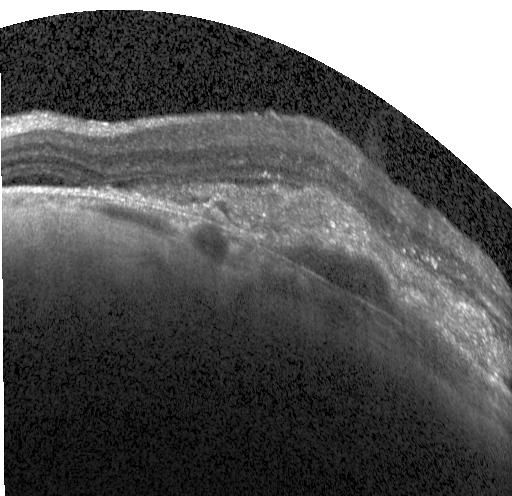

Retinal OCT cross-section. This B-scan demonstrates choroidal neovascularization.